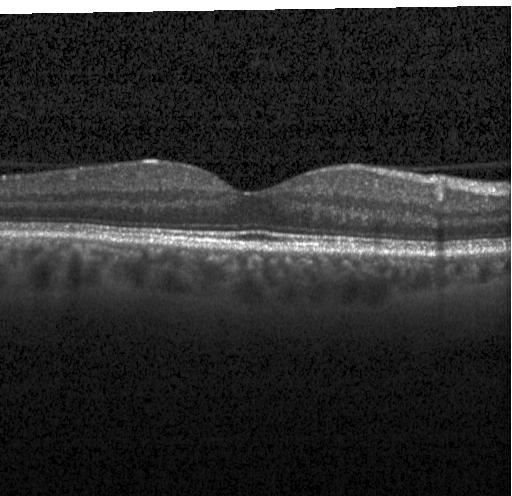
OCT line scan; macular scan; instrument: Heidelberg Spectralis.
The scan shows no CNV, no DME, and no drusen.